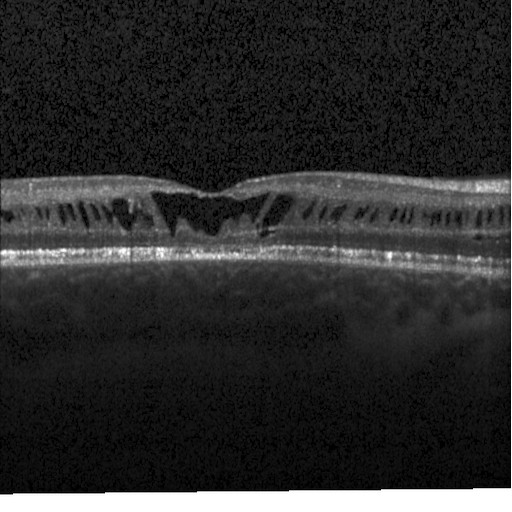

Instrument: Heidelberg Spectralis; SD-OCT; optical coherence tomography scan; fovea-centered. The scan shows diabetic macular edema (DME).